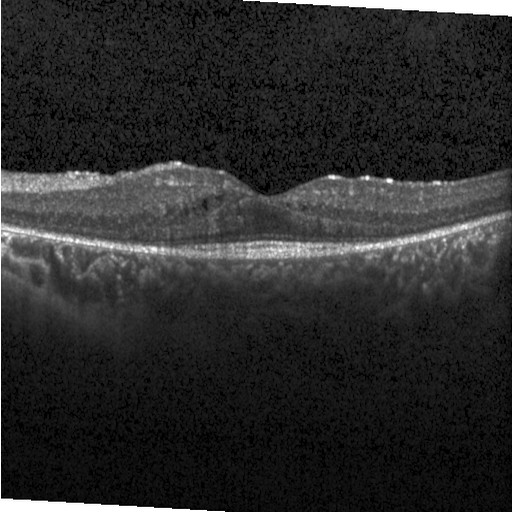

Macular OCT demonstrating diabetic macular edema.